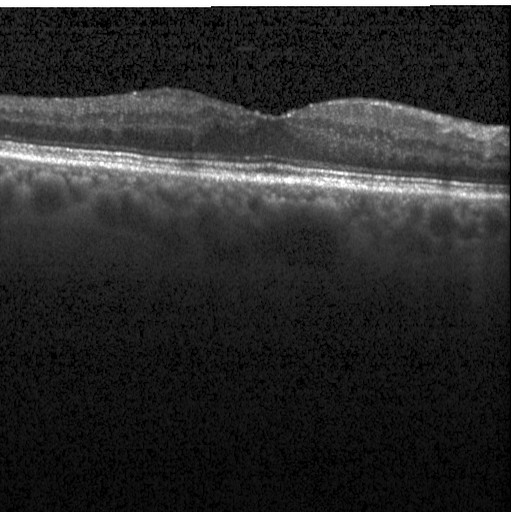
Finding: diabetic macular edema (DME).